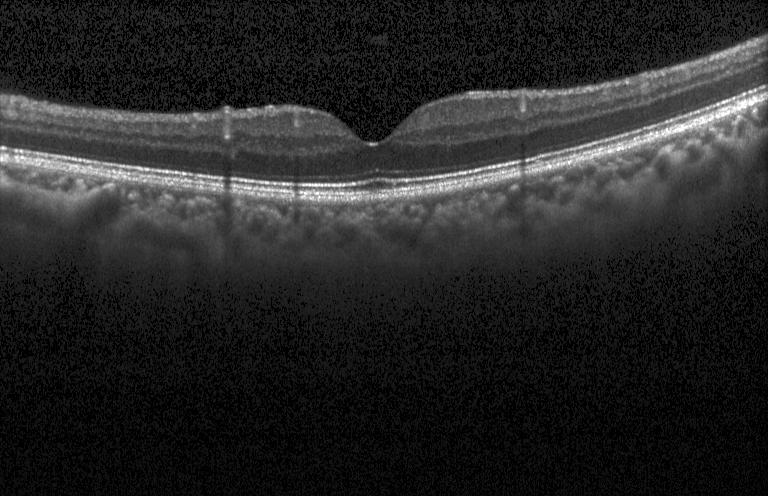
OCT B-scan; acquired on a Heidelberg Spectralis; spectral-domain optical coherence tomography; centered on the fovea
Finding: no evidence of choroidal neovascularization, diabetic macular edema, or drusen.